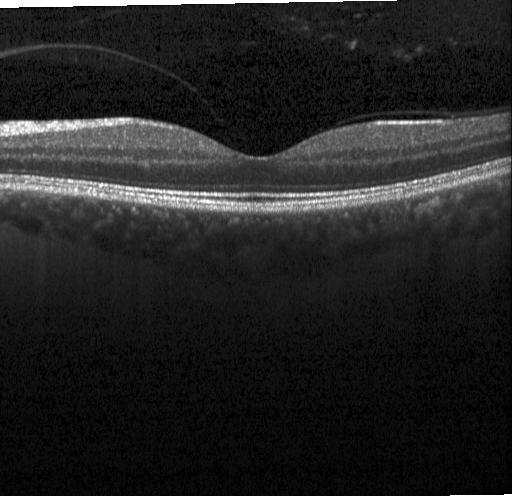
Spectral-domain optical coherence tomography · retinal OCT cross-section · Heidelberg Spectralis.
Diagnosis: neither choroidal neovascularization, diabetic macular edema, nor drusen.